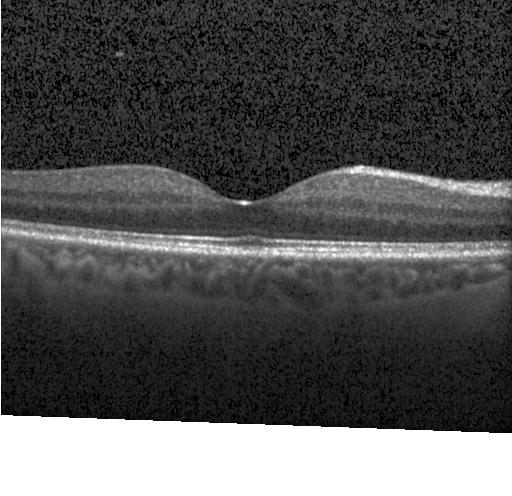
Acquired on a Heidelberg Spectralis; optical coherence tomography scan. Finding: no choroidal neovascularization, no diabetic macular edema, and no drusen.